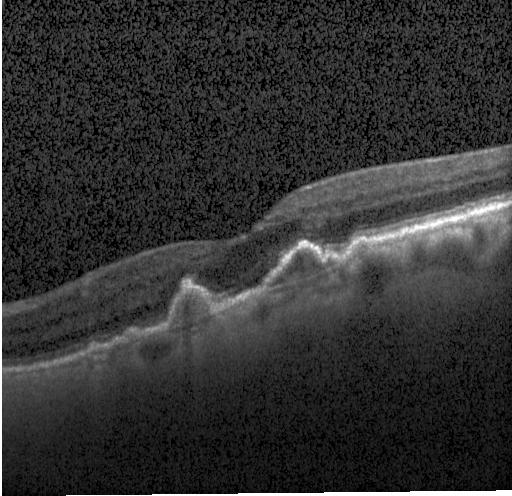
OCT line scan. Fovea-centered. SD-OCT. OCT finding: CNV.